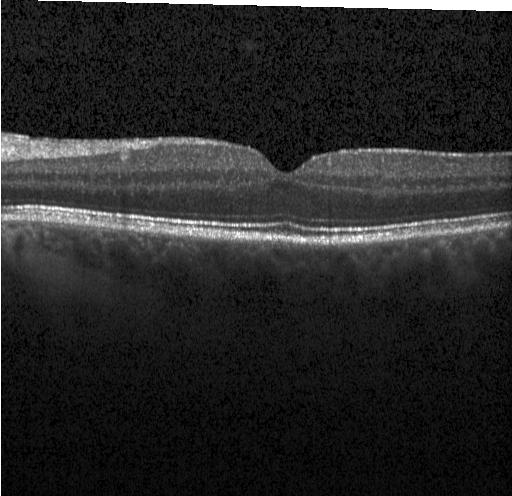

Optical coherence tomography scan. Instrument: Heidelberg Spectralis. Macular scan. No choroidal neovascularization, no diabetic macular edema, and no drusen.